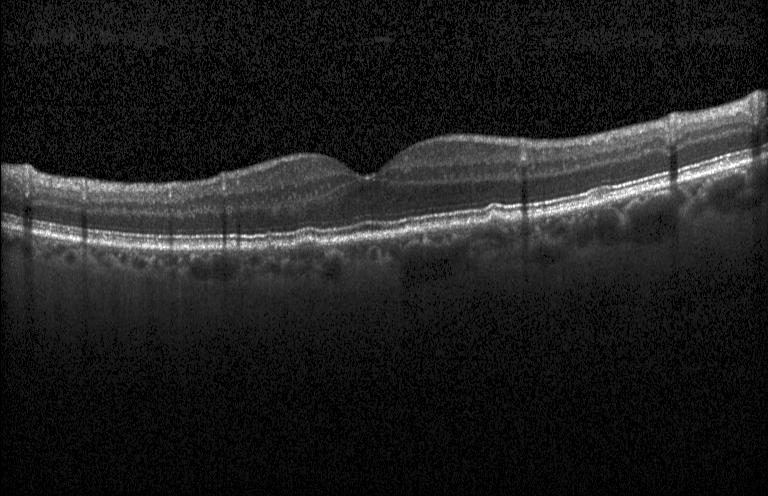 Fovea-centered, OCT line scan.
Dx: drusen.